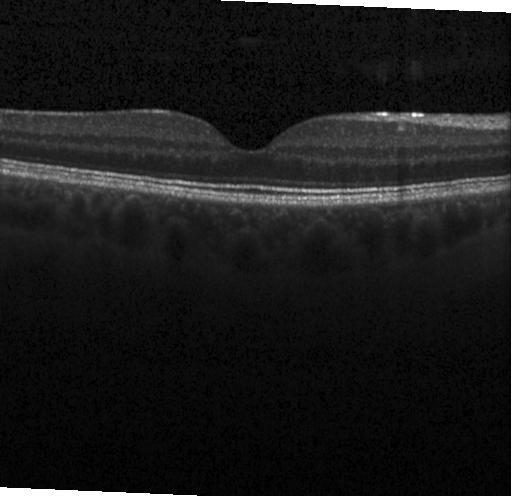 Impression: no evidence of CNV, DME, or drusen.